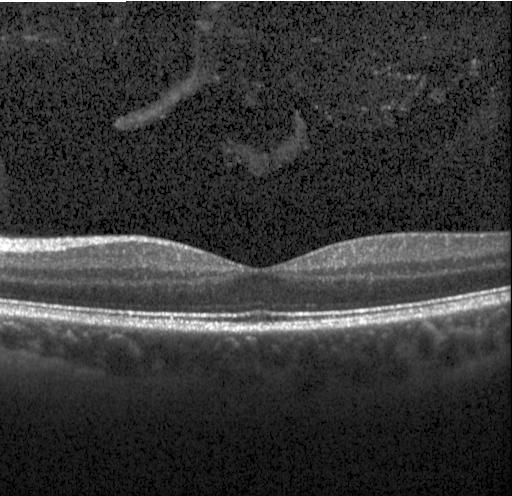

OCT line scan; horizontal scan through the fovea. Finding: neither choroidal neovascularization, diabetic macular edema, nor drusen.